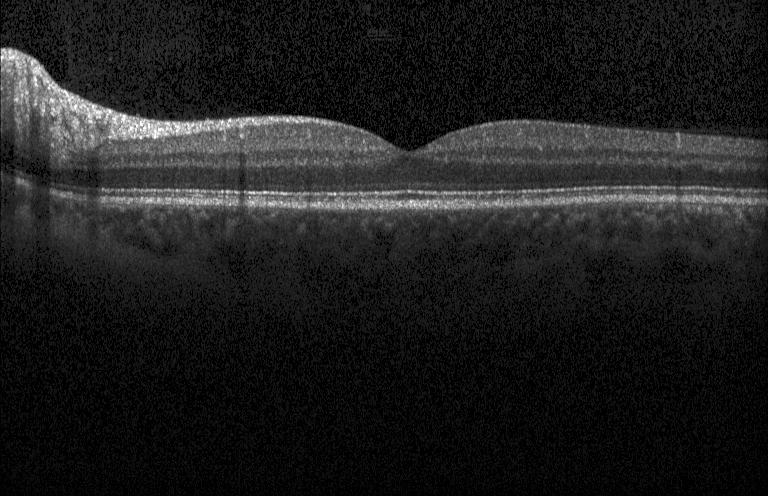

Fovea-centered. Acquired on a Heidelberg Spectralis. OCT line scan
Diagnosis: neither choroidal neovascularization, diabetic macular edema, nor drusen.